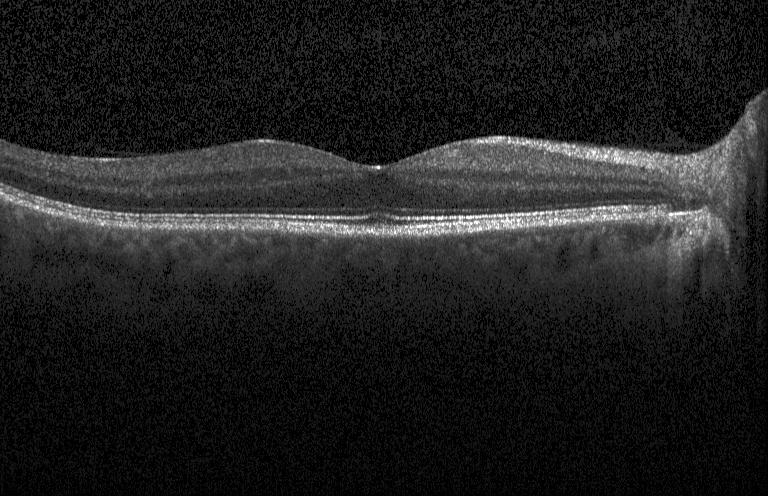
Optical coherence tomography B-scan · through the macula
This B-scan demonstrates neither choroidal neovascularization, diabetic macular edema, nor drusen.